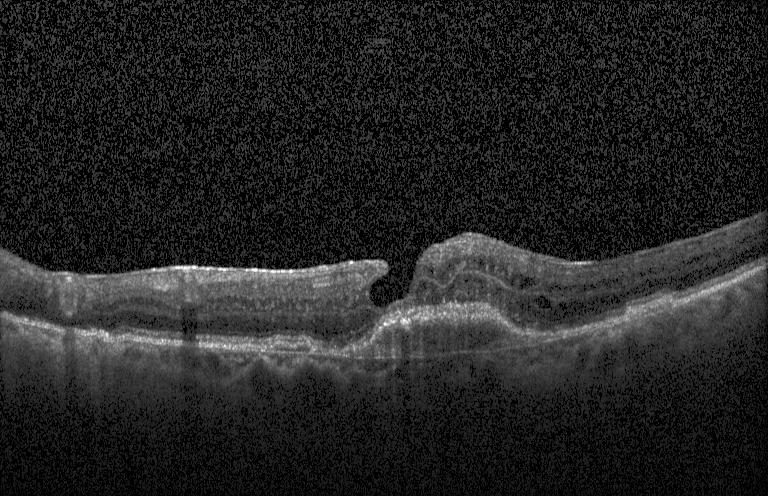

Spectral-domain optical coherence tomography, retinal OCT B-scan, fovea-centered. The scan shows choroidal neovascularization.